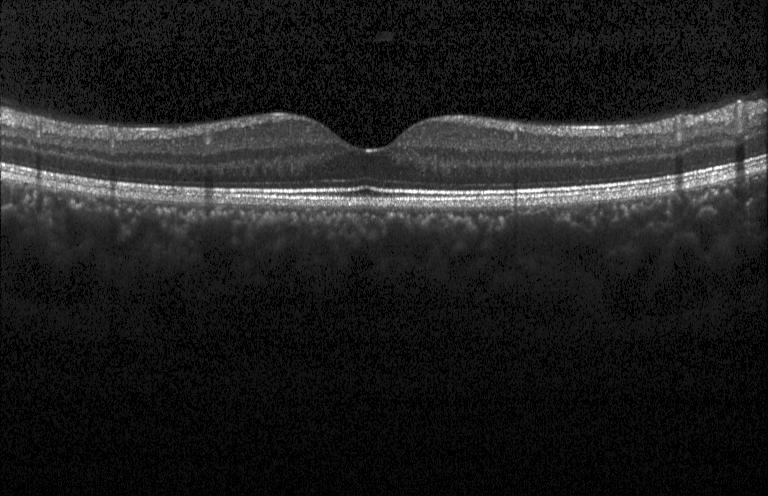
Centered on the fovea. Spectral-domain OCT. Optical coherence tomography scan. Assessment: no evidence of CNV, DME, or drusen.